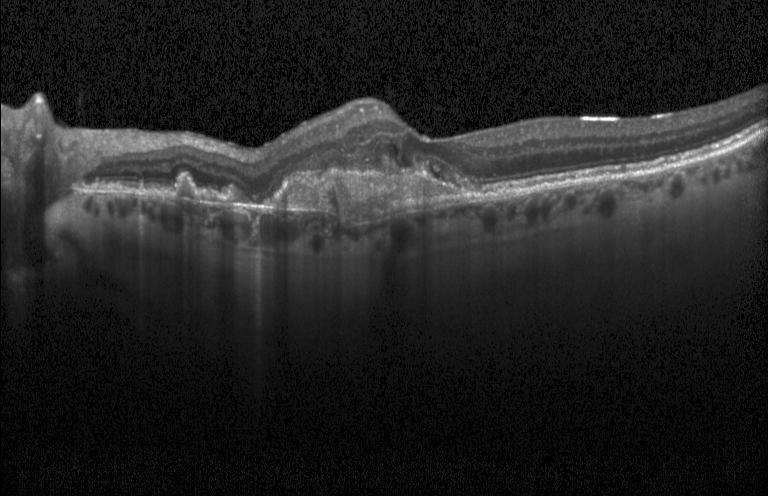 Retinal OCT B-scan
Impression: choroidal neovascularization.